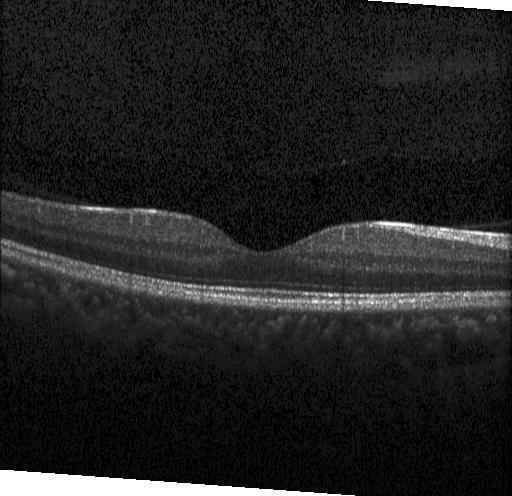
Retinal OCT B-scan — Macular OCT: no evidence of CNV, DME, or drusen.